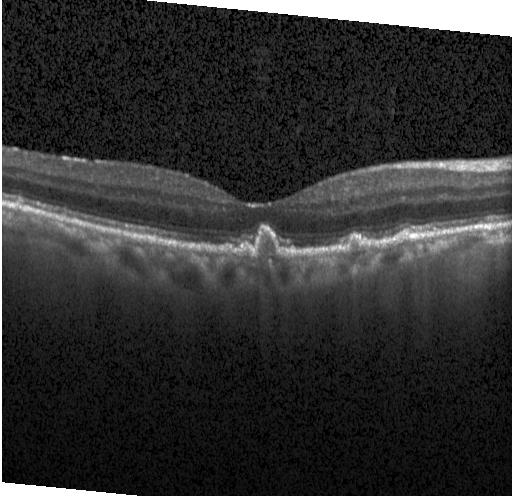 Spectral-domain optical coherence tomography, retinal OCT cross-section.
Multiple drusen.